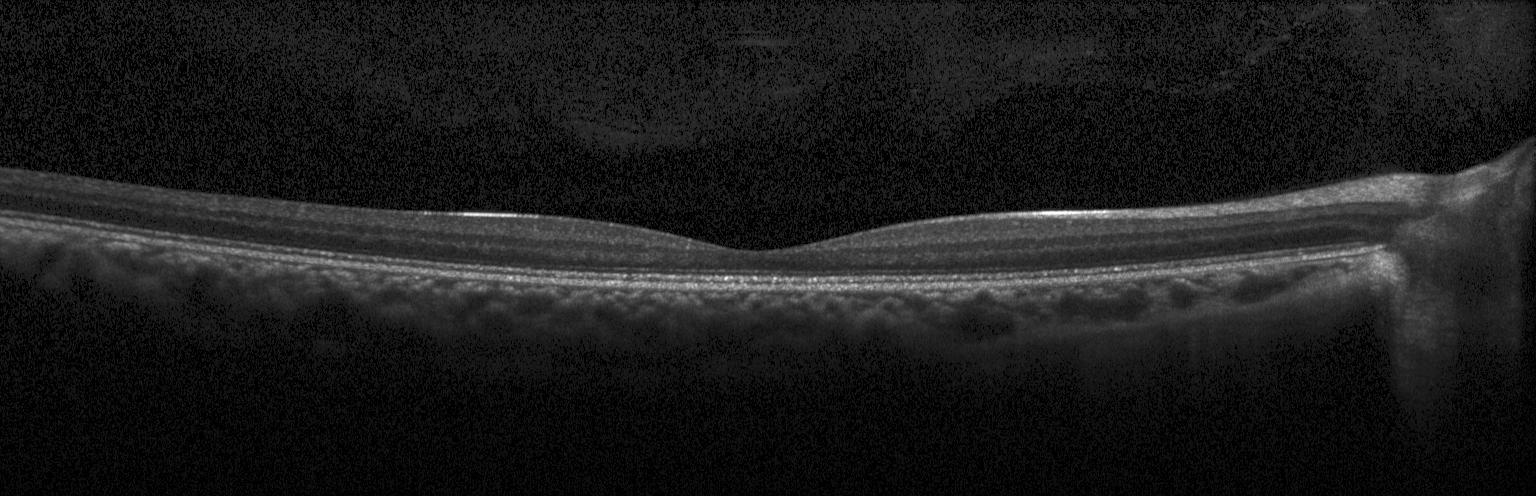
Heidelberg Spectralis OCT system, OCT line scan, spectral-domain optical coherence tomography.
Macular OCT: no choroidal neovascularization, diabetic macular edema, or drusen.